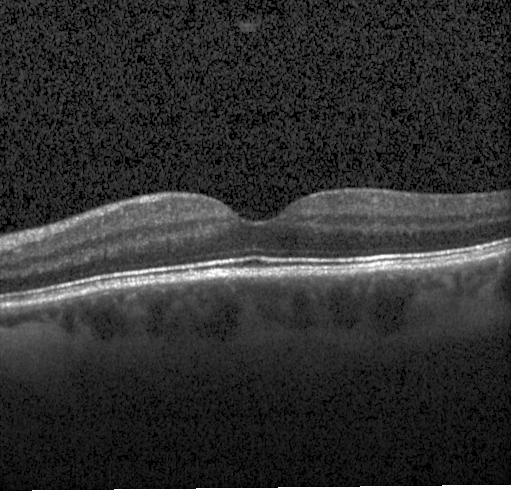
Diagnosis: no choroidal neovascularization, no diabetic macular edema, and no drusen.